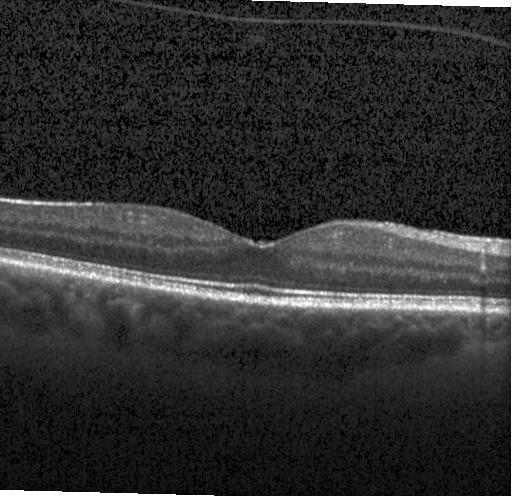 Spectral-domain optical coherence tomography · acquired on a Heidelberg Spectralis · OCT B-scan · centered on the fovea
Finding: no CNV, no DME, and no drusen.